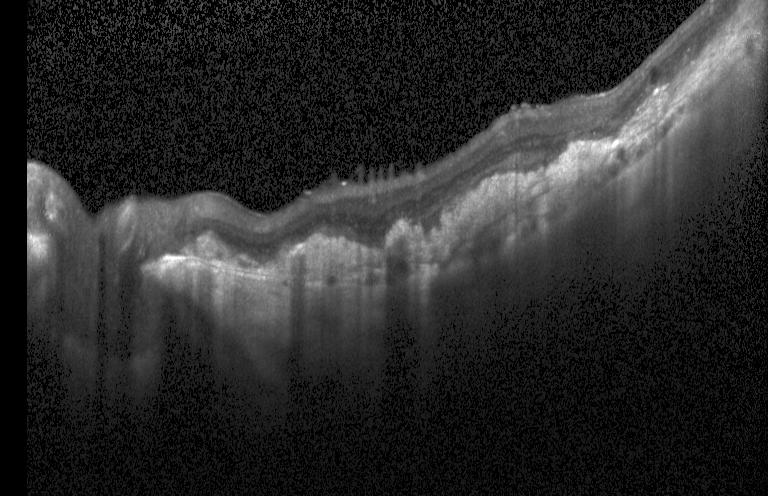
Retinal OCT cross-section · spectral-domain OCT
OCT finding: a choroidal neovascular membrane.